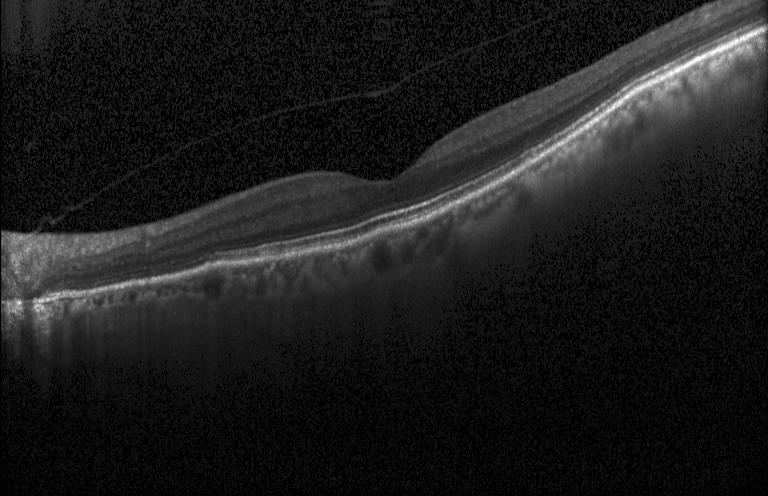
OCT B-scan — Impression: neither choroidal neovascularization, diabetic macular edema, nor drusen.